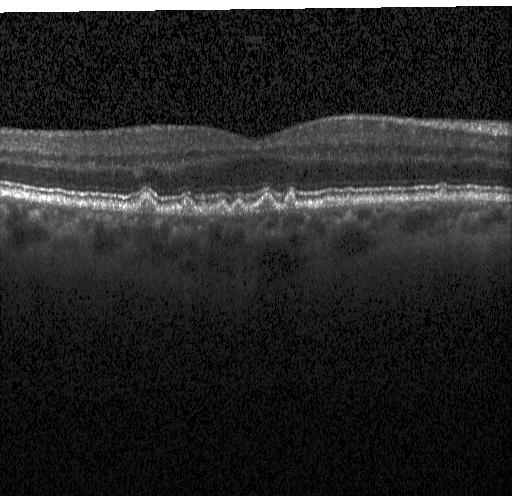 Acquired on a Heidelberg Spectralis, OCT line scan.
Diagnosis: drusen.